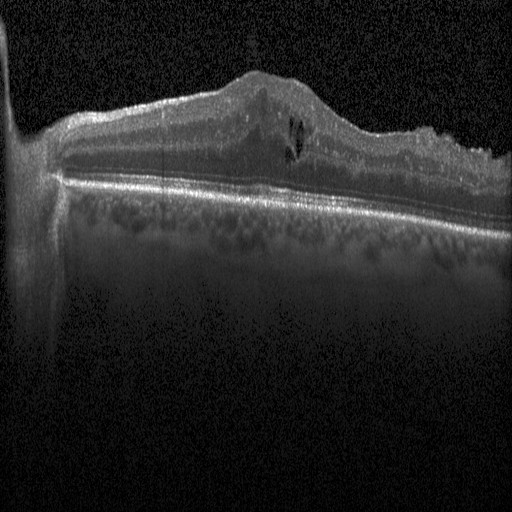

Retinal OCT cross-section; instrument: Heidelberg Spectralis — Macular OCT: DME.